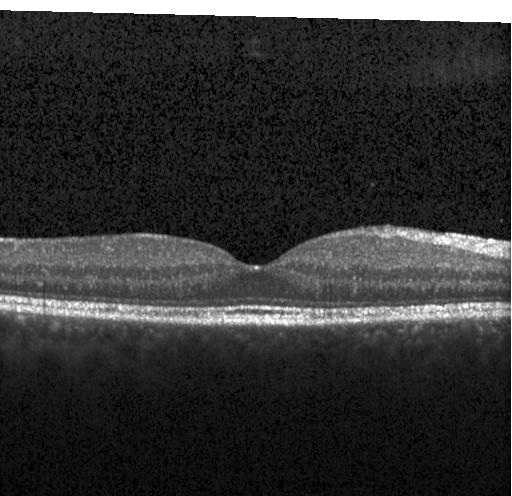
OCT finding: no evidence of choroidal neovascularization, diabetic macular edema, or drusen.